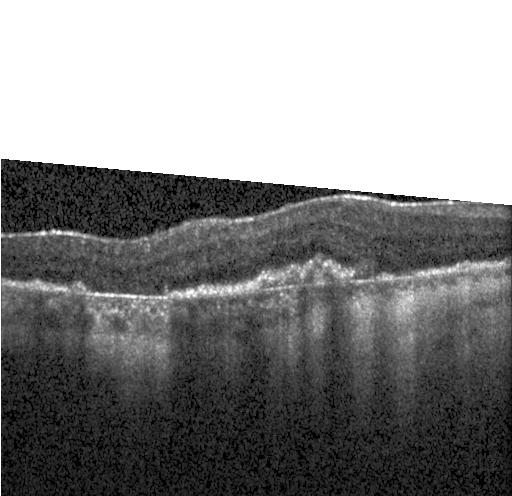 CNV.